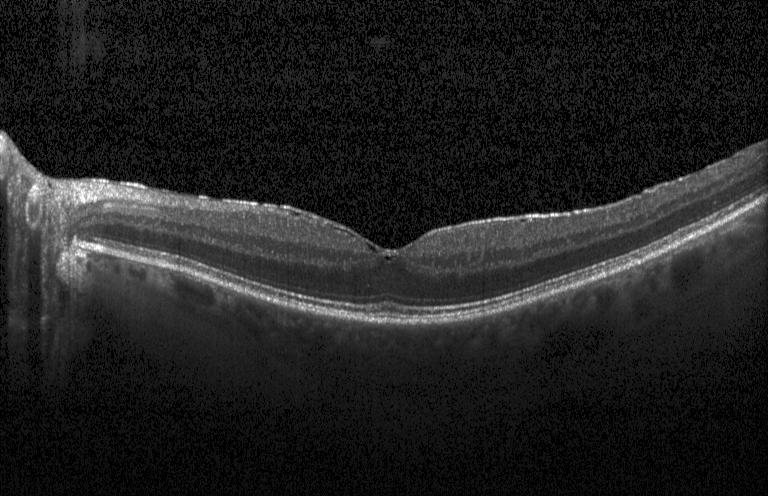 OCT line scan — Finding: no evidence of CNV, DME, or drusen.